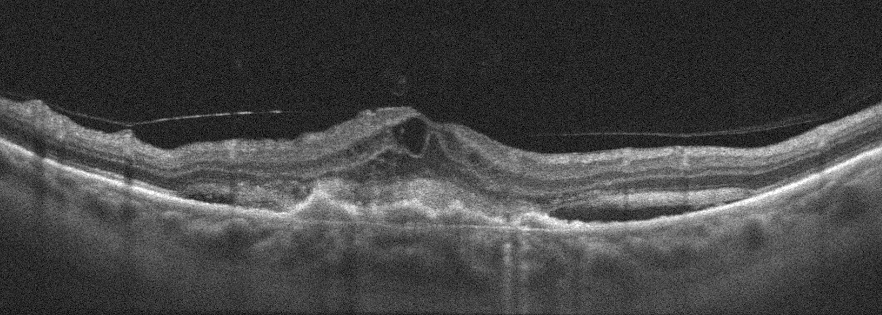 OCT line scan, macular scan, left eye — This B-scan demonstrates age-related macular degeneration.